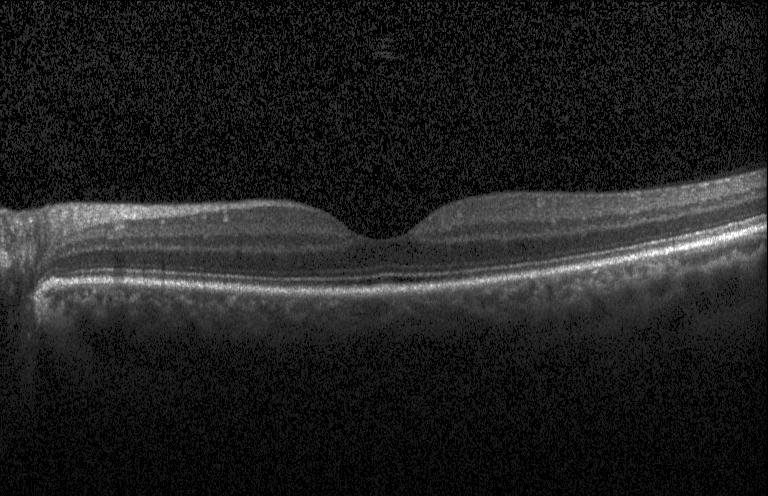
Spectral-domain optical coherence tomography. OCT line scan. Fovea-centered. Acquired on a Heidelberg Spectralis
The scan shows no evidence of choroidal neovascularization, diabetic macular edema, or drusen.